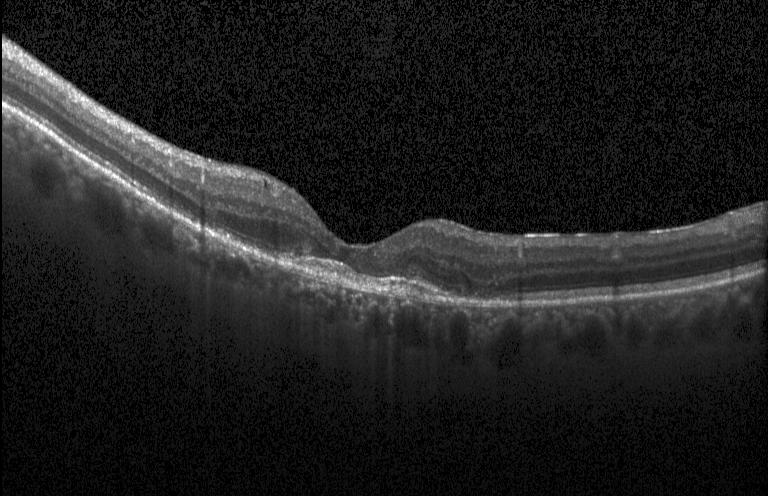

Spectral-domain OCT, Heidelberg Spectralis OCT system, optical coherence tomography scan
The scan shows a choroidal neovascular membrane.